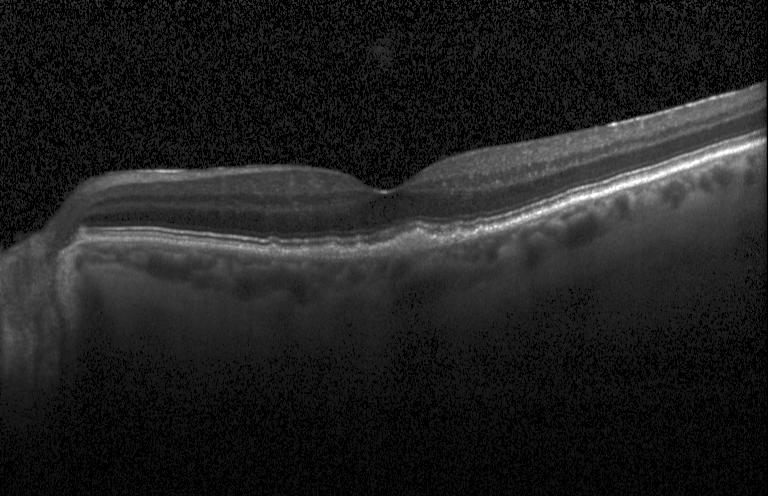 Optical coherence tomography B-scan. Drusen.